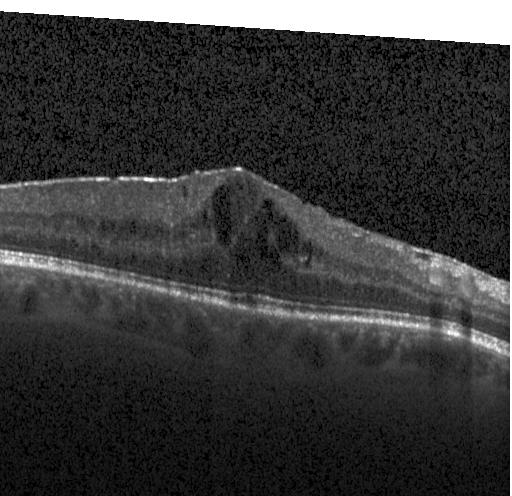
OCT scan showing diabetic macular edema (DME).